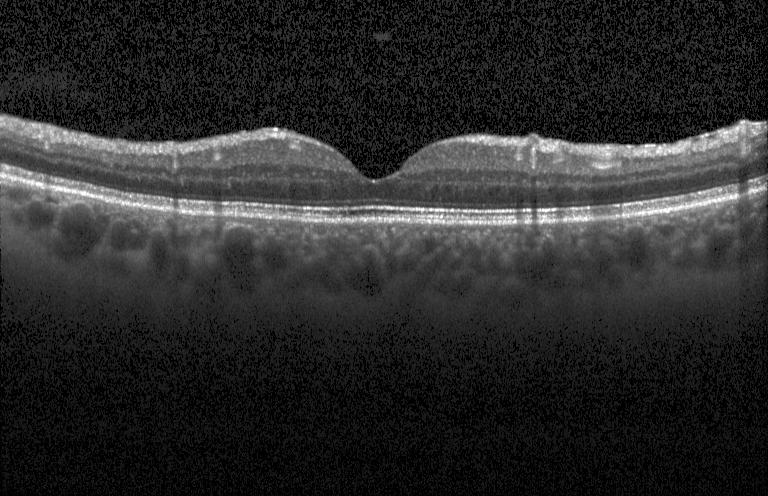
Optical coherence tomography B-scan; Heidelberg Spectralis; spectral-domain optical coherence tomography; horizontal scan through the fovea. Impression: no choroidal neovascularization, diabetic macular edema, or drusen.